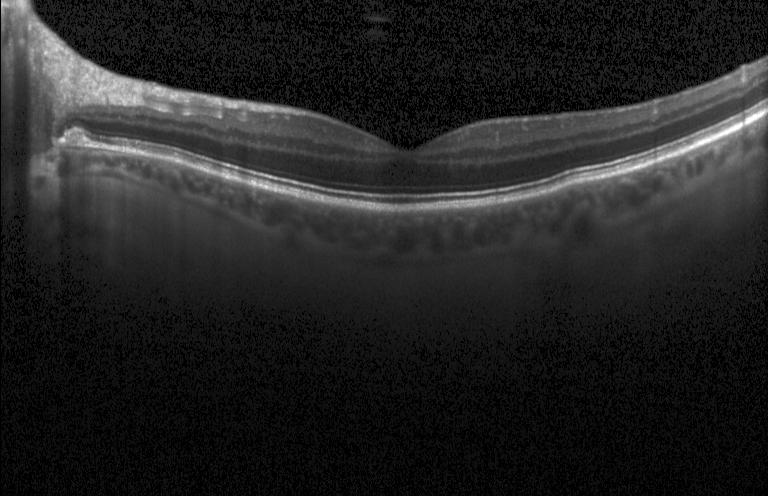
The scan shows no choroidal neovascularization, diabetic macular edema, or drusen.